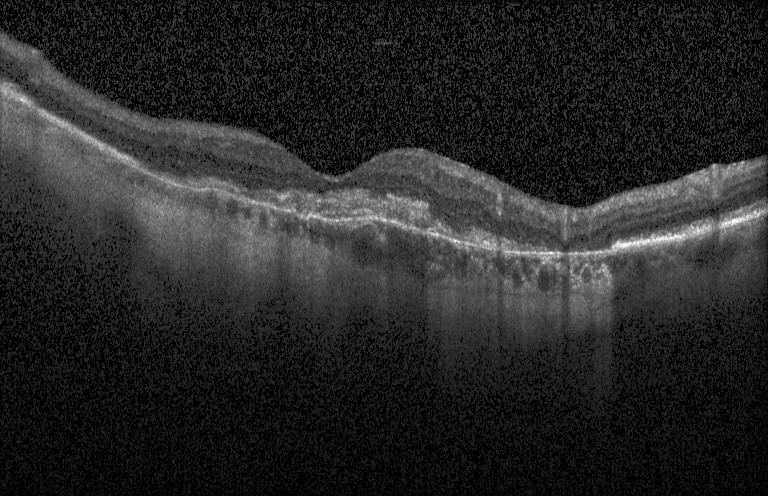 A choroidal neovascular membrane.